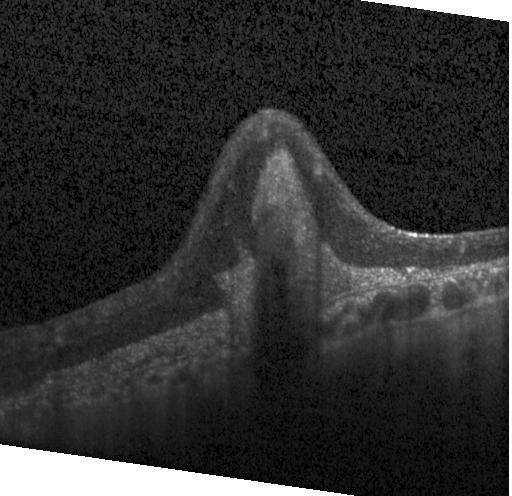

Optical coherence tomography scan
CNV.